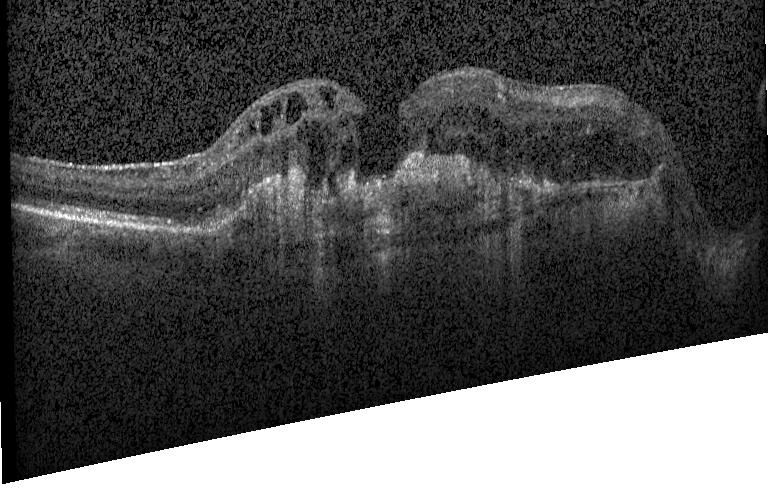 Spectral-domain OCT; optical coherence tomography B-scan. Diagnosis: a choroidal neovascular membrane.